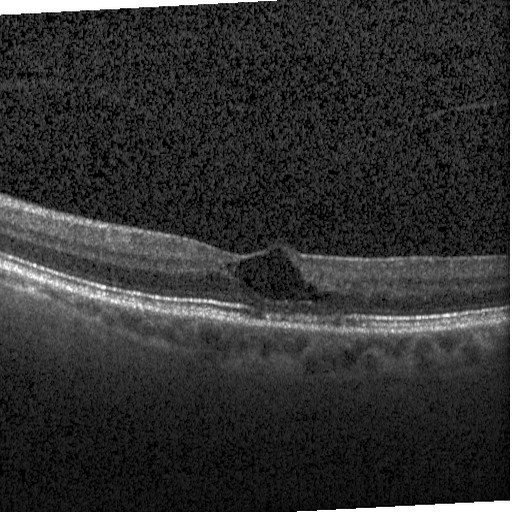

OCT finding: DME.